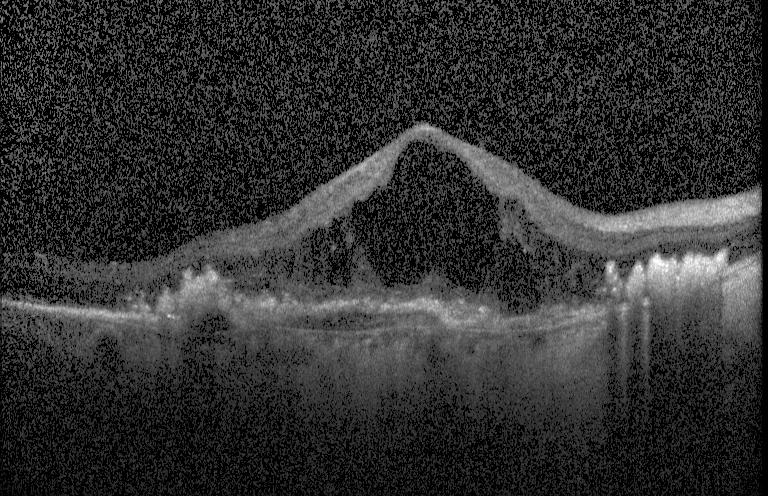
Fovea-centered, OCT line scan.
Dx: a choroidal neovascular membrane.